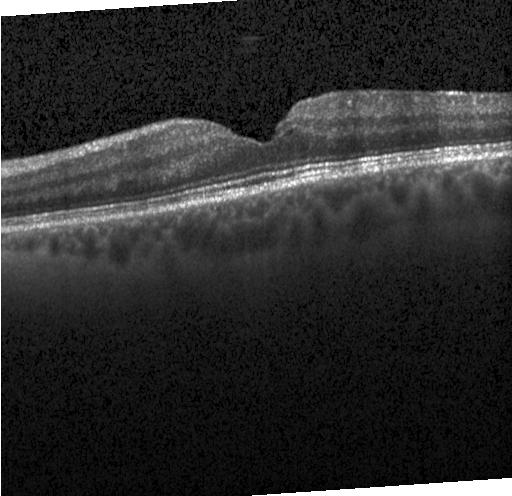

SD-OCT; optical coherence tomography B-scan; horizontal scan through the fovea; instrument: Heidelberg Spectralis — Diagnosis: neither CNV, DME, nor drusen.